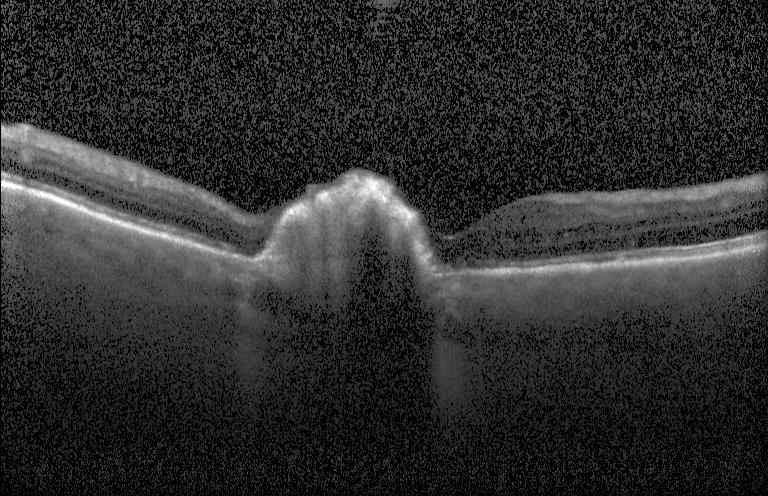

Optical coherence tomography scan. Finding: a choroidal neovascular membrane.